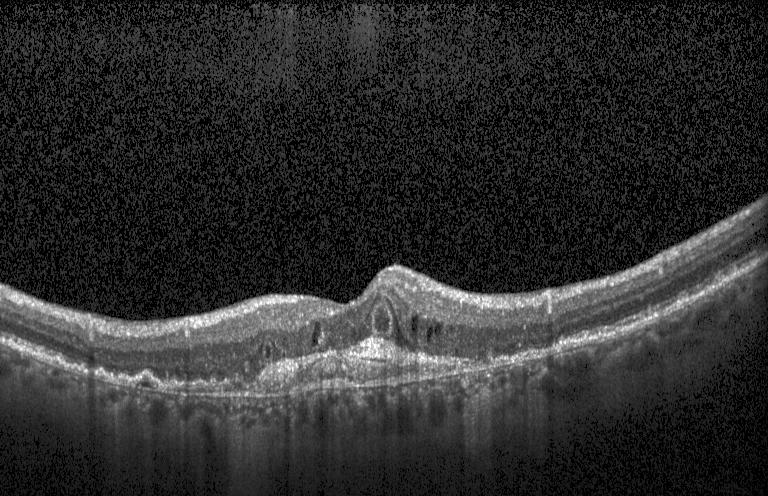
Spectral-domain OCT B-scan: choroidal neovascularization.